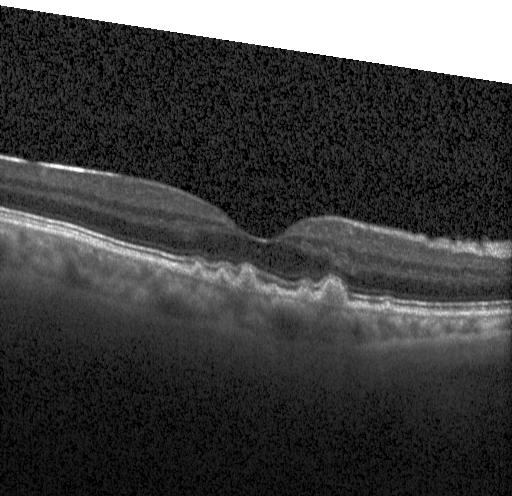

SD-OCT · optical coherence tomography scan
Assessment: drusen.